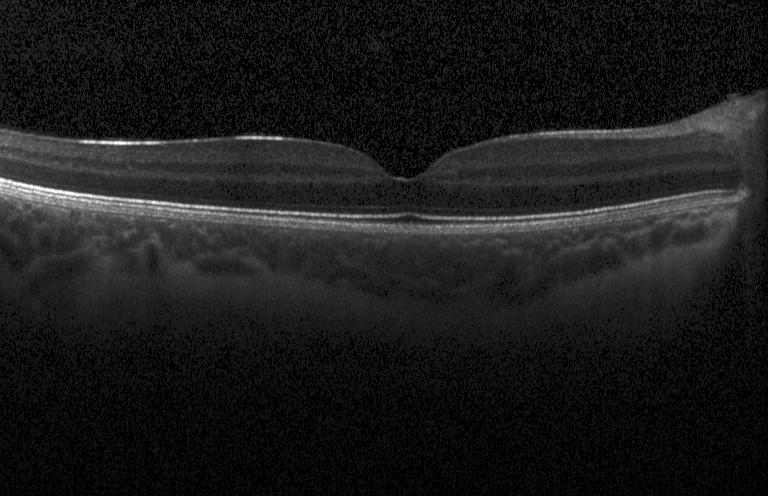

Retinal OCT B-scan. Macular scan. Impression: no choroidal neovascularization, no diabetic macular edema, and no drusen.